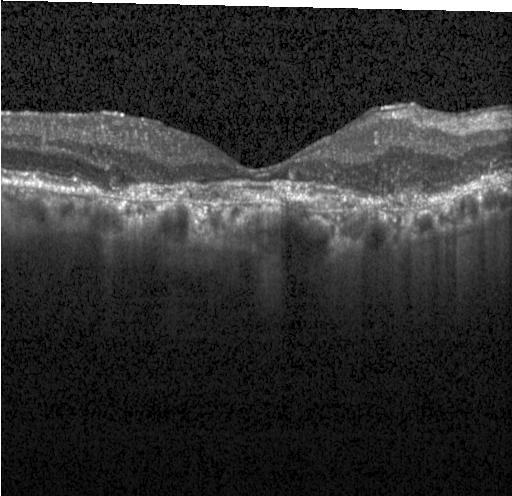
OCT scan showing CNV.